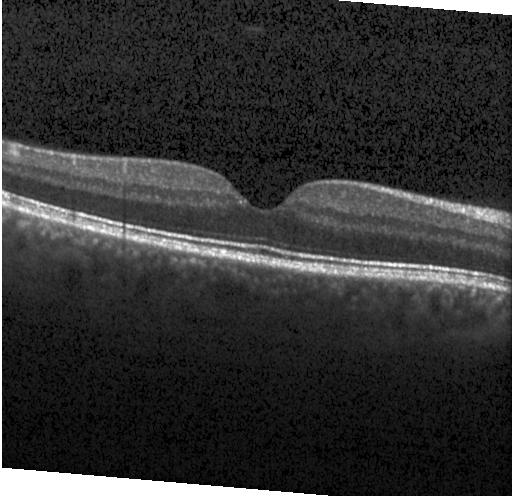

Optical coherence tomography scan. No CNV, no DME, and no drusen.